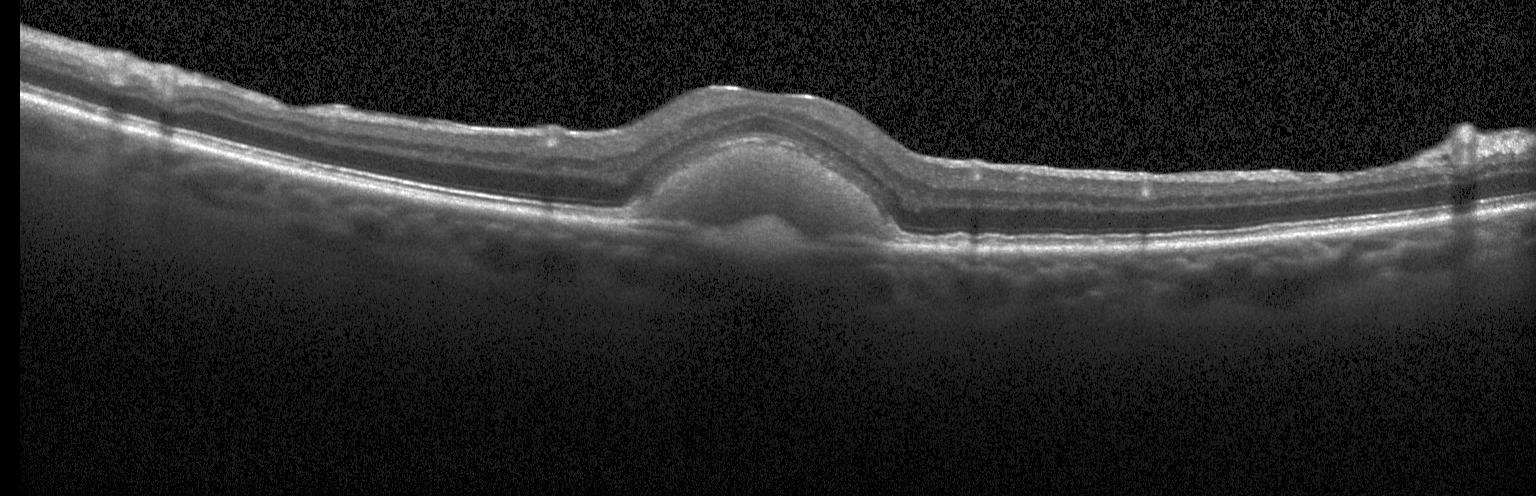
Optical coherence tomography scan · instrument: Heidelberg Spectralis. Diagnosis: choroidal neovascularization (CNV).